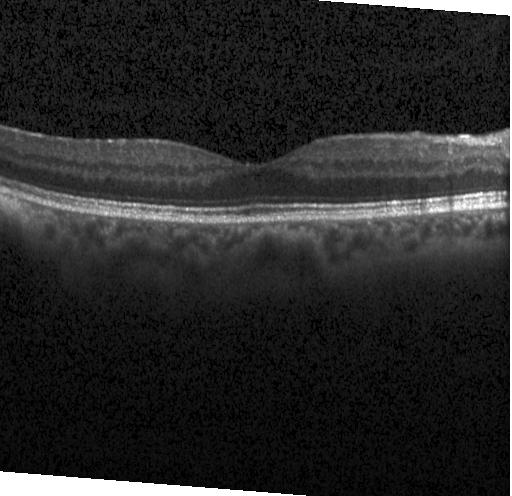

SD-OCT, Heidelberg Spectralis, centered on the fovea, OCT B-scan
Macular OCT: no choroidal neovascularization, diabetic macular edema, or drusen.